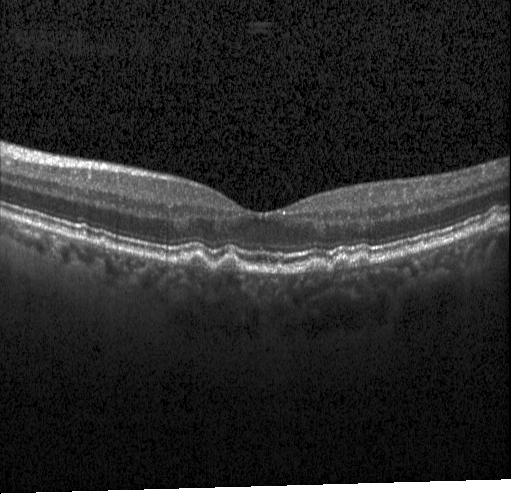

This B-scan demonstrates drusen.